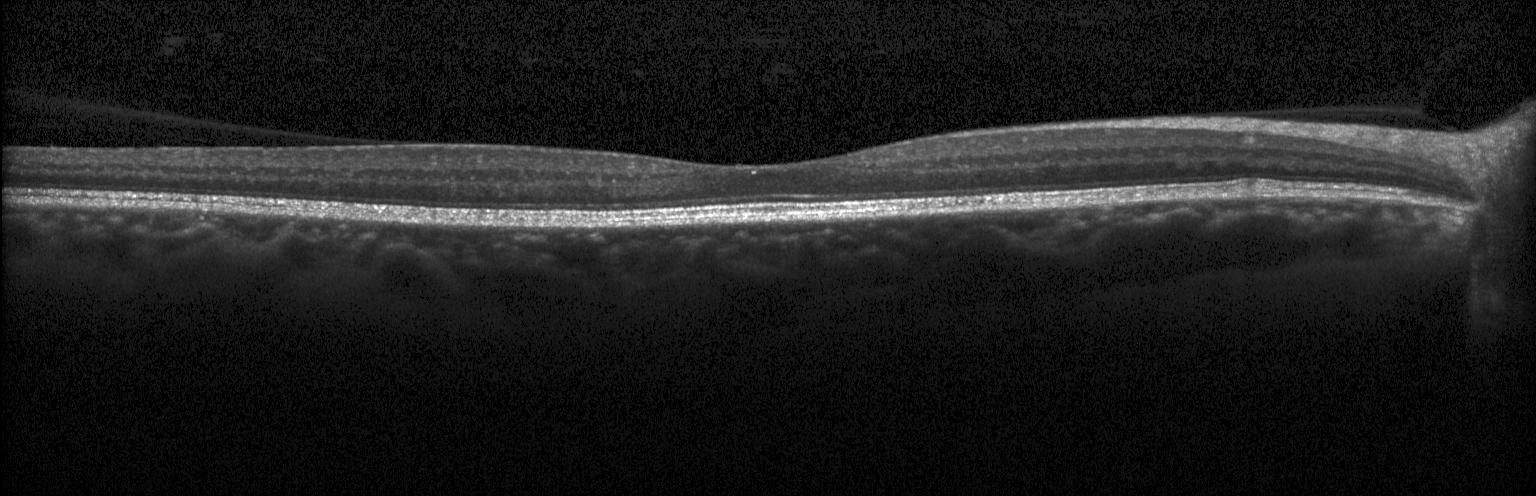

OCT B-scan, spectral-domain optical coherence tomography, fovea-centered
Diagnosis: neither CNV, DME, nor drusen.